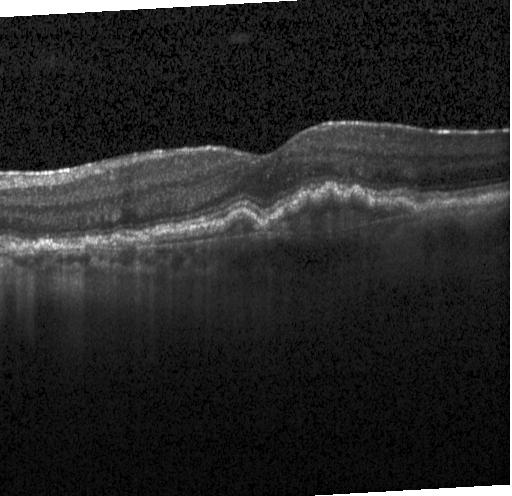 CNV.